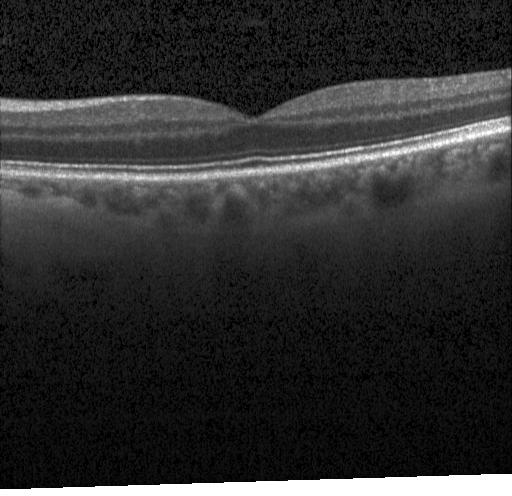 Optical coherence tomography scan, spectral-domain optical coherence tomography. Diagnosis: no choroidal neovascularization, no diabetic macular edema, and no drusen.